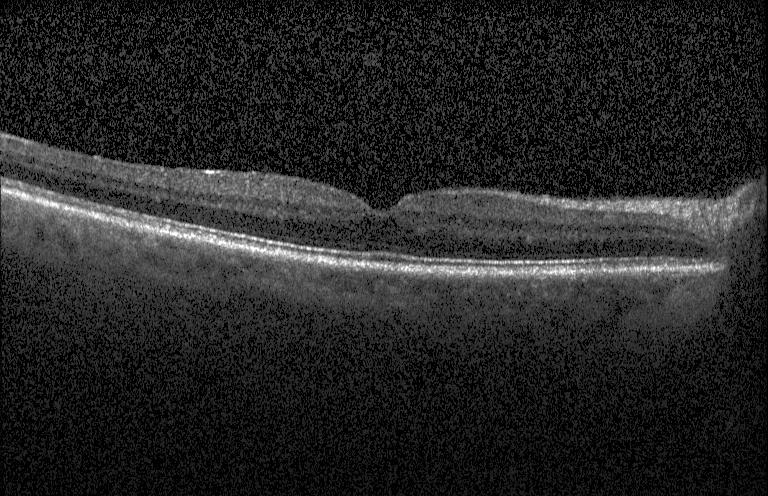 OCT finding: no CNV, DME, or drusen.